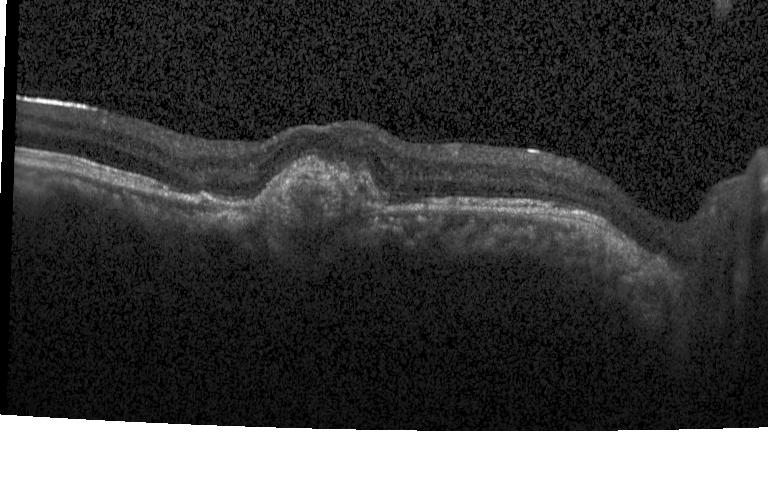

Diagnosis: a choroidal neovascular membrane.